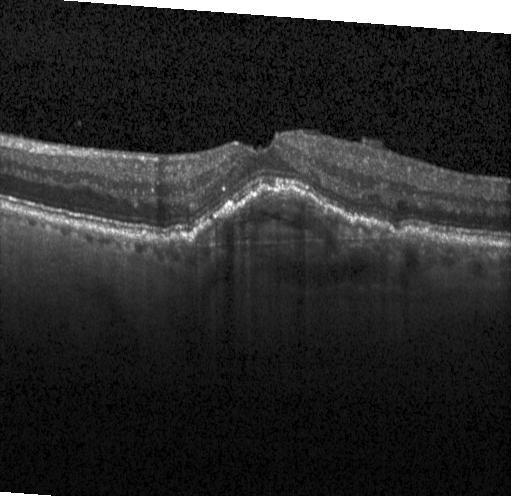 Retinal OCT B-scan
Dx: choroidal neovascularization (CNV).